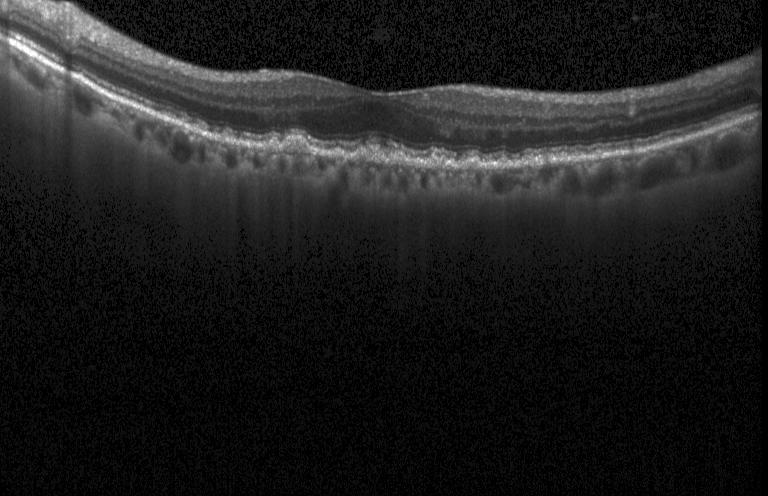
SD-OCT. Retinal OCT cross-section.
Impression: multiple drusen.